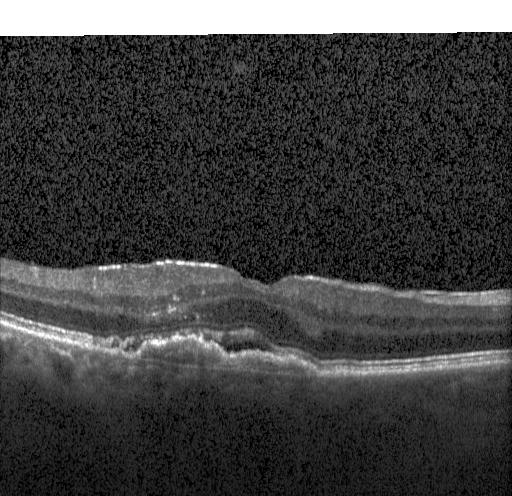
Heidelberg Spectralis OCT system; centered on the fovea; OCT line scan; SD-OCT. Assessment: CNV.